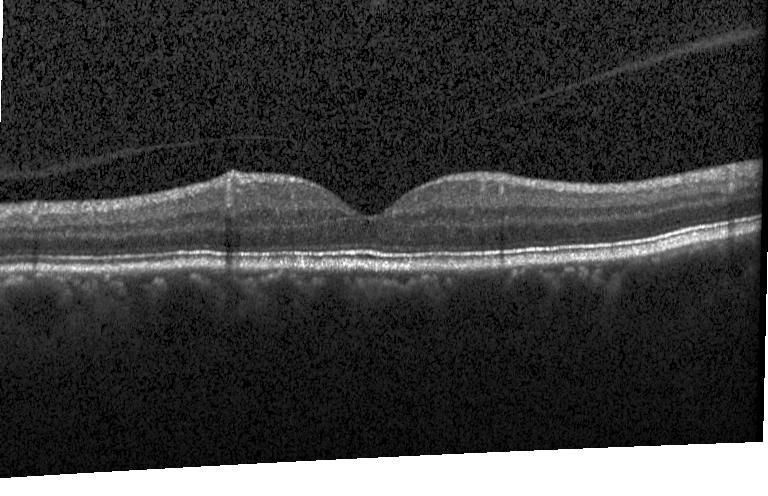 Through the macula; spectral-domain OCT; Heidelberg Spectralis; optical coherence tomography B-scan — Impression: no evidence of choroidal neovascularization, diabetic macular edema, or drusen.